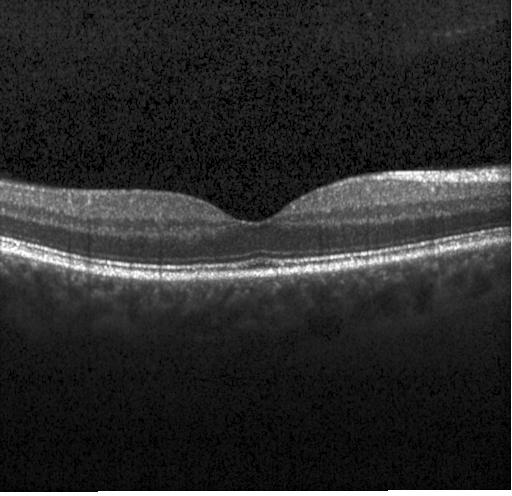

Macular scan. Acquired on a Heidelberg Spectralis. Optical coherence tomography B-scan — OCT finding: neither choroidal neovascularization, diabetic macular edema, nor drusen.